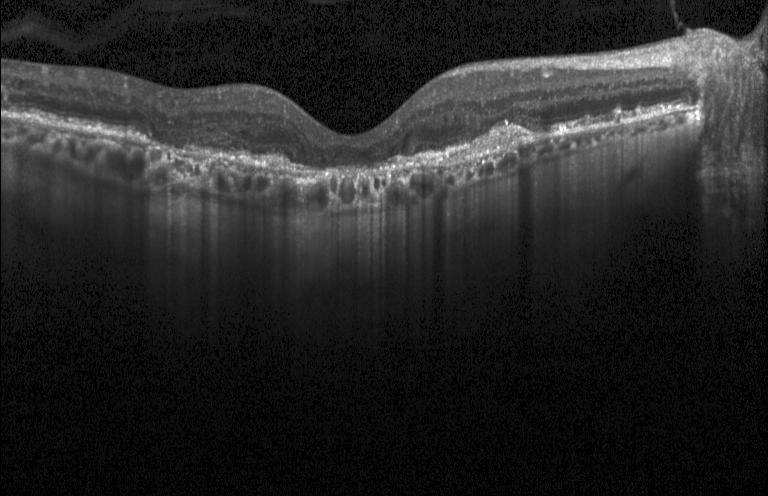 Instrument: Heidelberg Spectralis · spectral-domain OCT · optical coherence tomography B-scan
Diagnosis: choroidal neovascularization.